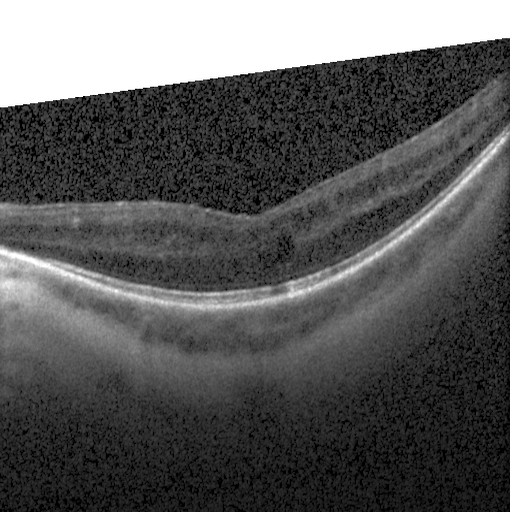

Instrument: Heidelberg Spectralis · fovea-centered · optical coherence tomography scan · spectral-domain optical coherence tomography
Impression: diabetic macular edema.